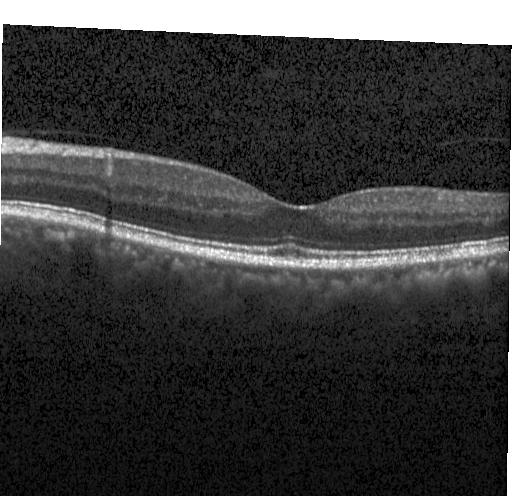 OCT B-scan showing no CNV, no DME, and no drusen.